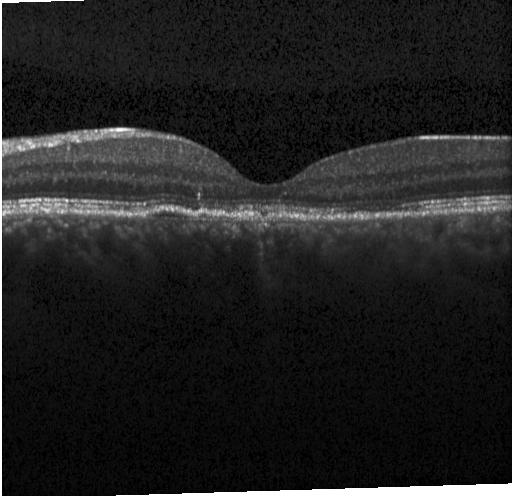

Through the macula. Retinal OCT cross-section. Acquired on a Heidelberg Spectralis. Spectral-domain optical coherence tomography.
Impression: multiple drusen.